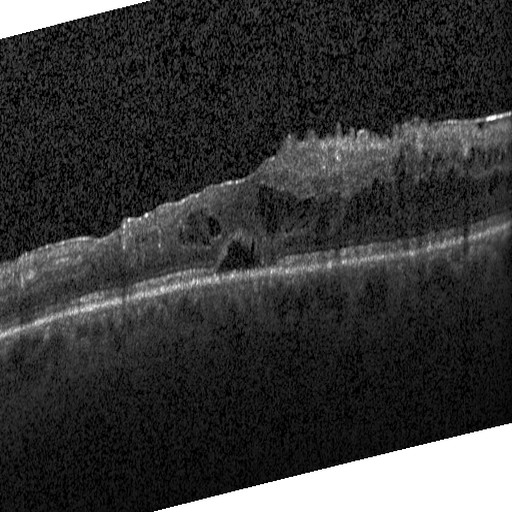
Assessment: diabetic macular edema.